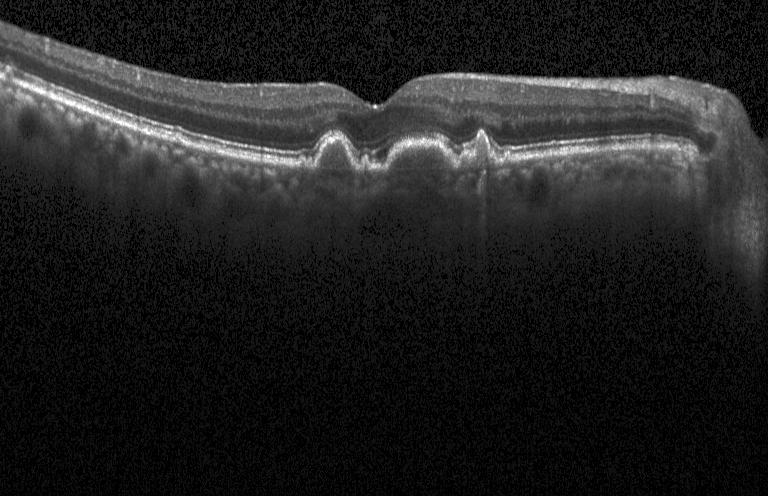 OCT line scan. Diagnosis: multiple drusen.